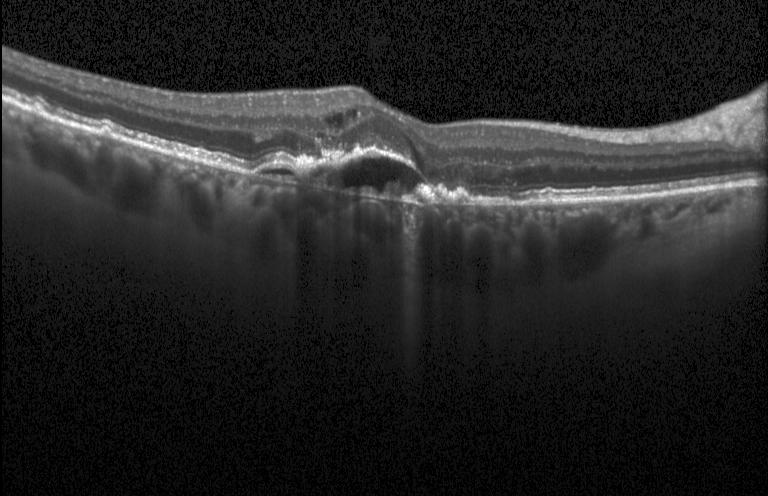
Optical coherence tomography B-scan · through the macula. This B-scan demonstrates a choroidal neovascular membrane.